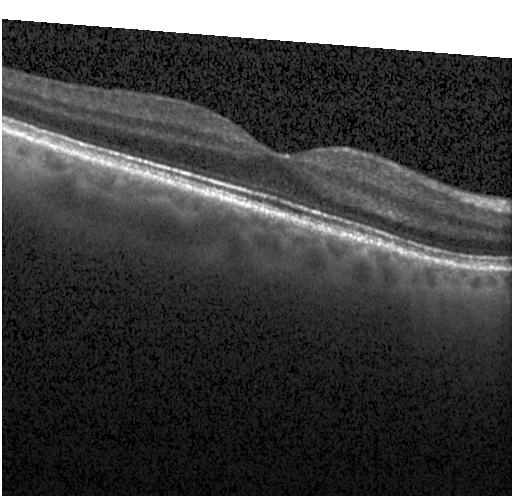 The scan shows no evidence of CNV, DME, or drusen.